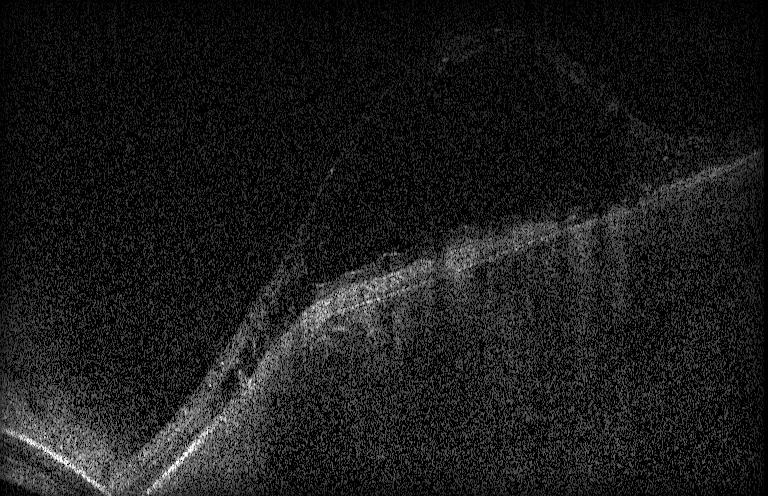 SD-OCT. Through the macula. OCT B-scan. Acquired on a Heidelberg Spectralis.
Finding: a choroidal neovascular membrane.